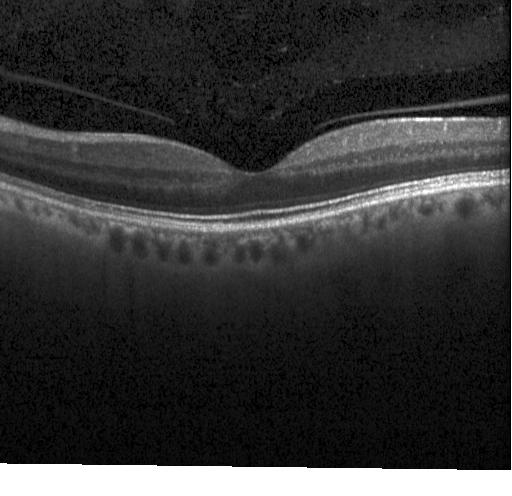 Finding: no evidence of choroidal neovascularization, diabetic macular edema, or drusen.